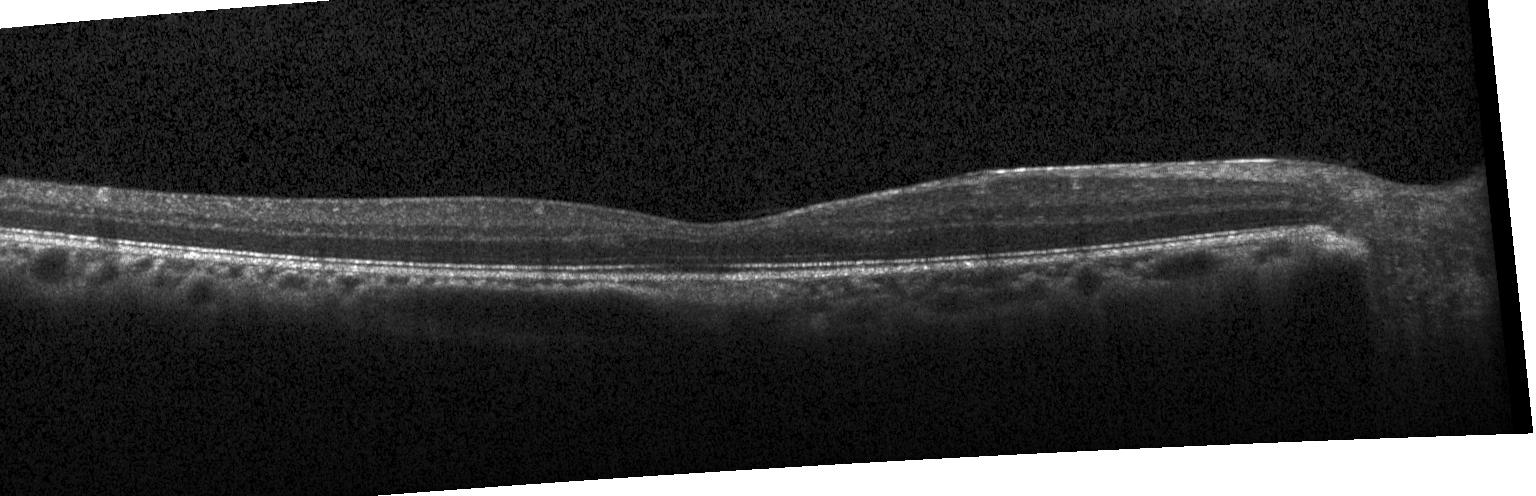 Spectral-domain optical coherence tomography, OCT line scan, acquired on a Heidelberg Spectralis — Diagnosis: no CNV, DME, or drusen.